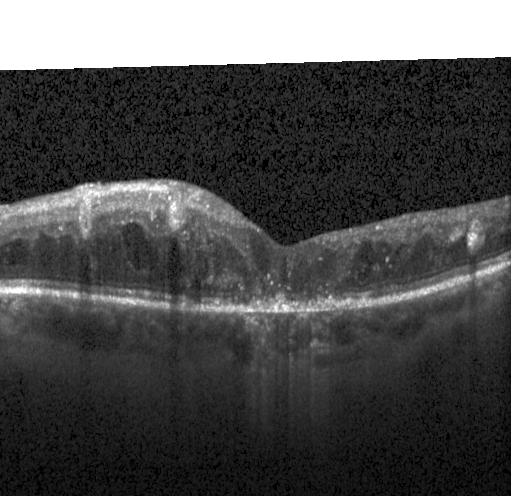
Heidelberg Spectralis. Retinal OCT cross-section. Spectral-domain OCT. Fovea-centered. Impression: diabetic macular edema (DME).